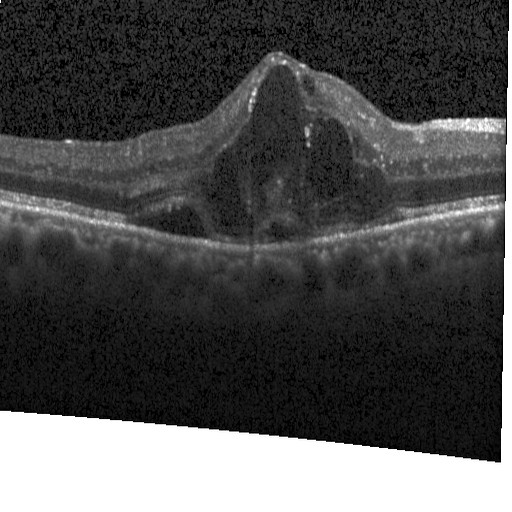
Fovea-centered, OCT B-scan, spectral-domain optical coherence tomography.
Diabetic macular edema.